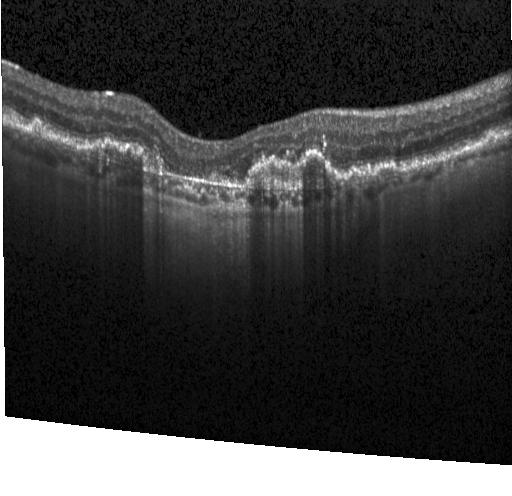

A choroidal neovascular membrane.